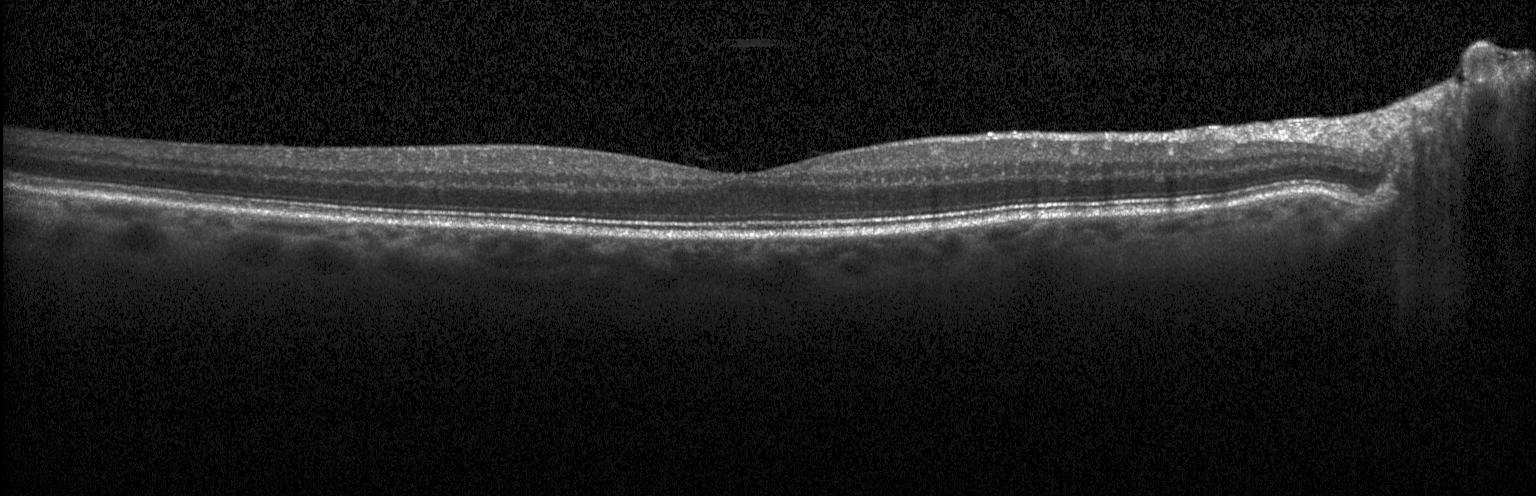

Spectral-domain OCT · through the macula · OCT line scan.
Finding: no CNV, no DME, and no drusen.